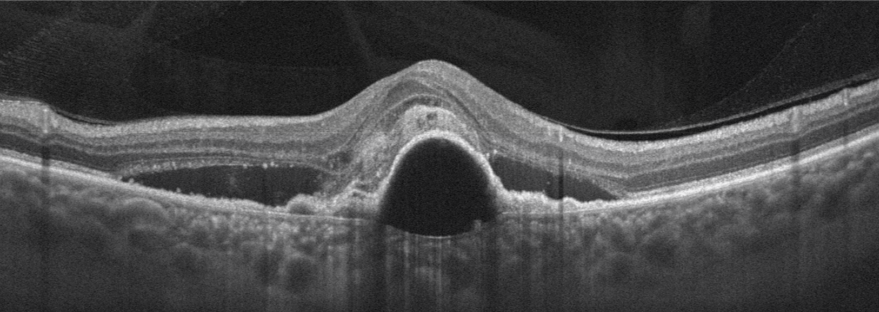 Optovue Avanti RTVue XR · OCT B-scan · macular scan — Dx: age-related macular degeneration (AMD).